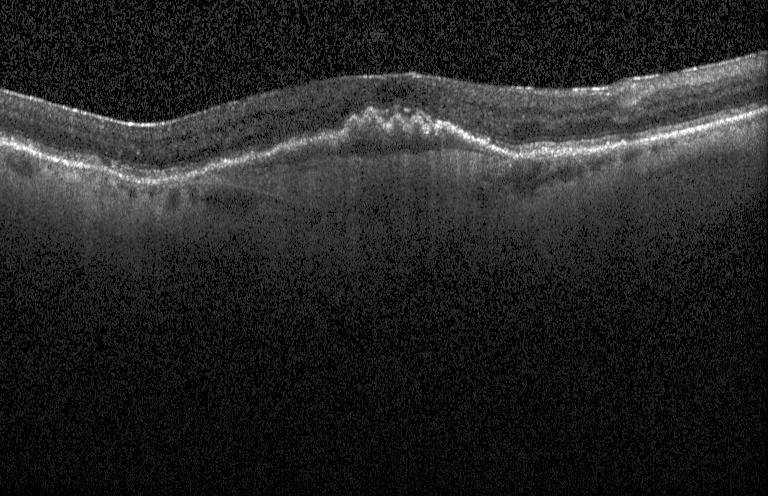 The scan shows a choroidal neovascular membrane.